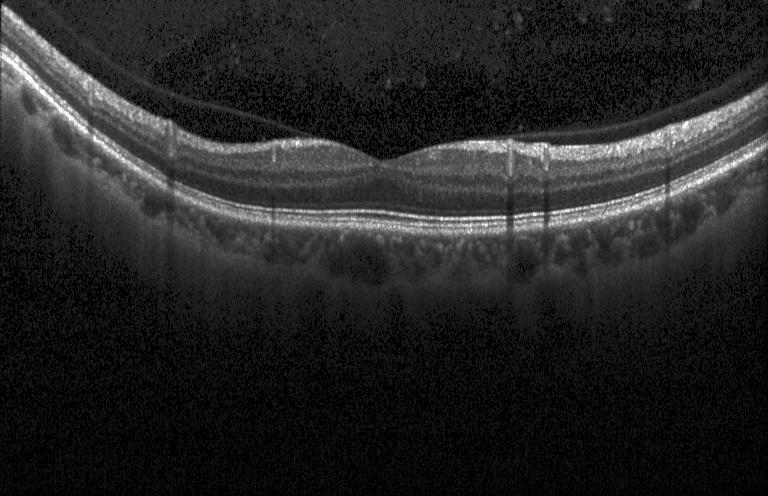
Centered on the fovea, SD-OCT, OCT line scan. Diagnosis: neither choroidal neovascularization, diabetic macular edema, nor drusen.